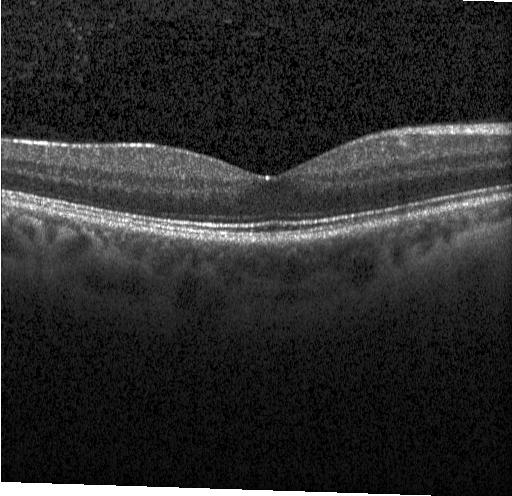
Optical coherence tomography B-scan; Heidelberg Spectralis; centered on the fovea; spectral-domain OCT — Impression: no choroidal neovascularization, no diabetic macular edema, and no drusen.